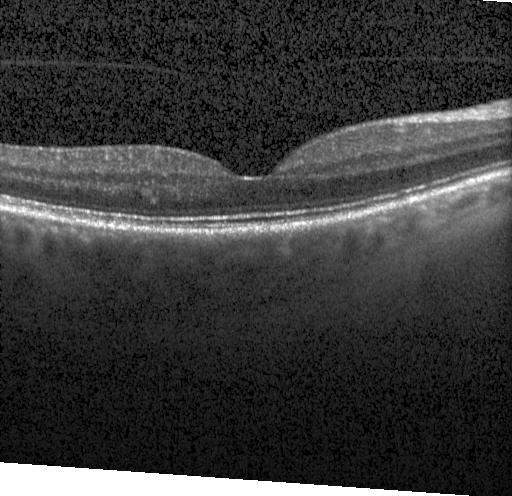

Retinal OCT B-scan · horizontal scan through the fovea · Heidelberg Spectralis · spectral-domain optical coherence tomography. Impression: no evidence of choroidal neovascularization, diabetic macular edema, or drusen.